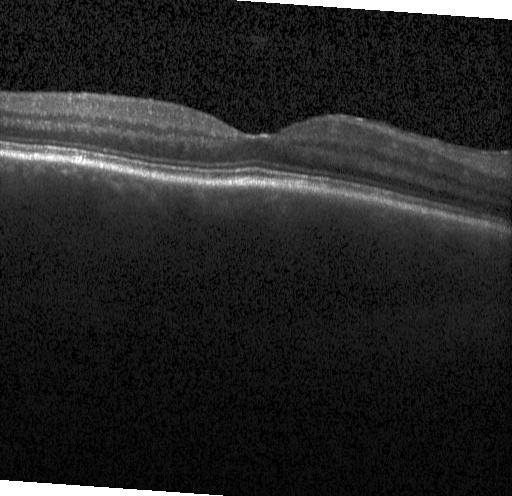 Retinal OCT B-scan, spectral-domain OCT — Dx: no choroidal neovascularization, diabetic macular edema, or drusen.